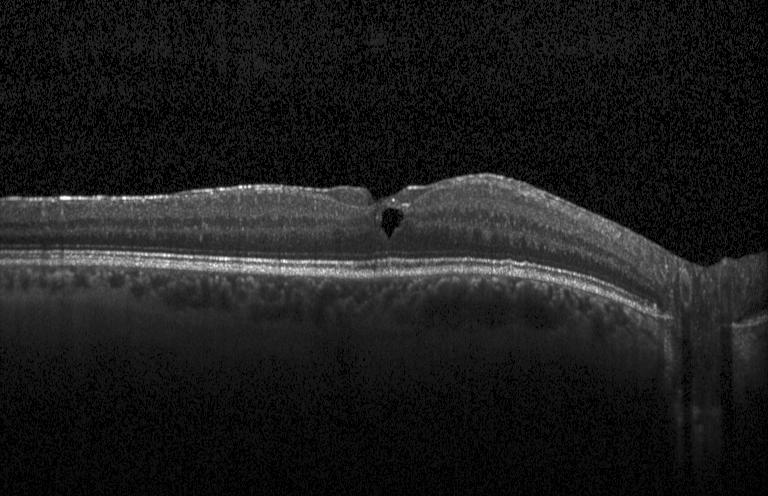

SD-OCT. Optical coherence tomography B-scan. Instrument: Heidelberg Spectralis
Diagnosis: diabetic macular edema (DME).